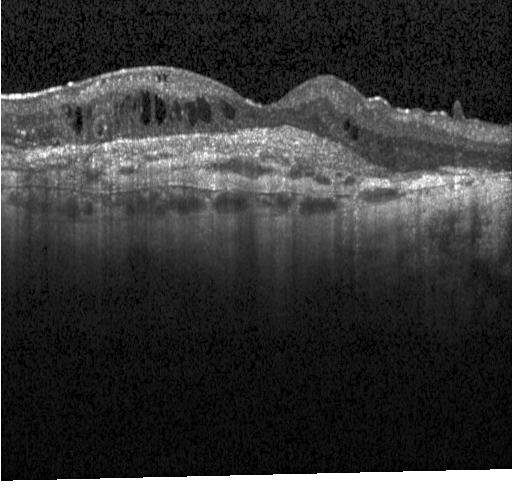
OCT scan showing CNV.